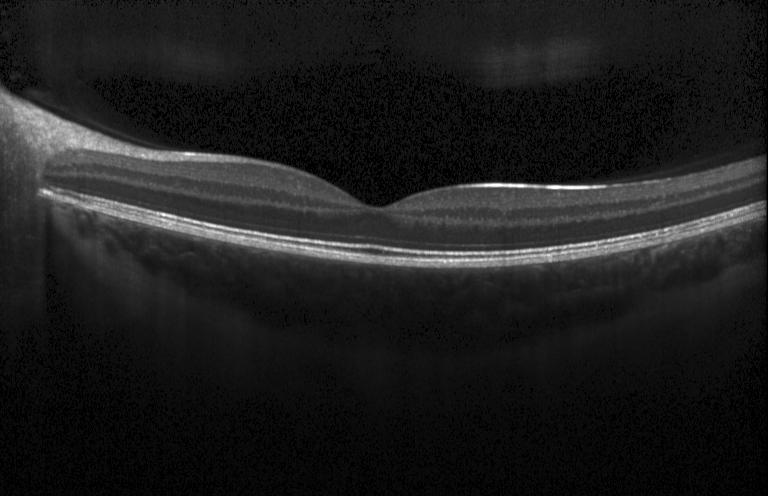

Retinal OCT cross-section. Dx: no choroidal neovascularization, no diabetic macular edema, and no drusen.